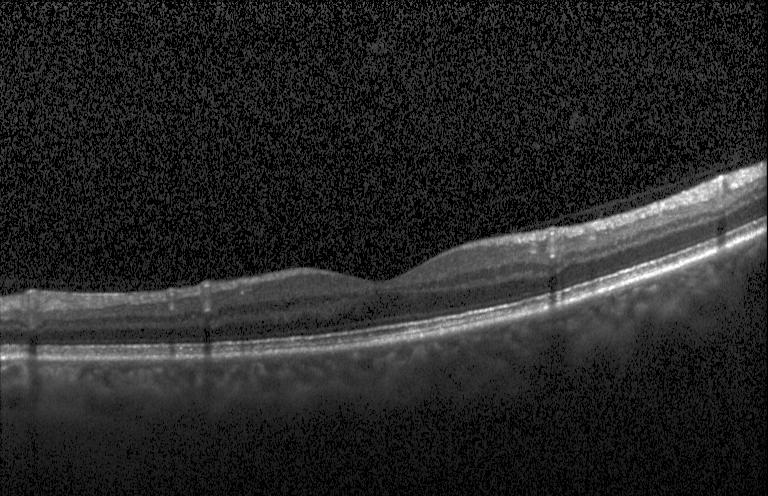
Macular scan · optical coherence tomography B-scan — Macular OCT: no choroidal neovascularization, diabetic macular edema, or drusen.